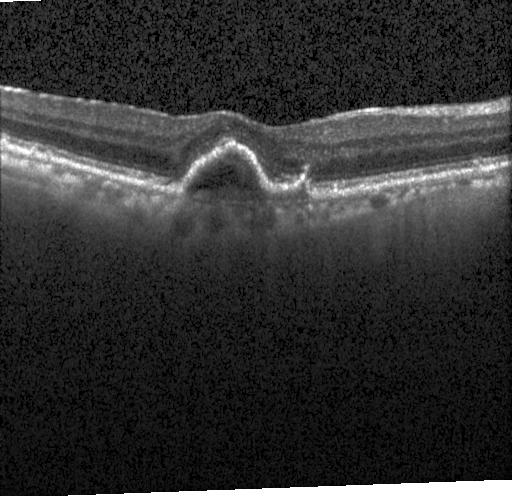 Macular scan · spectral-domain OCT · OCT B-scan — This B-scan demonstrates choroidal neovascularization (CNV).